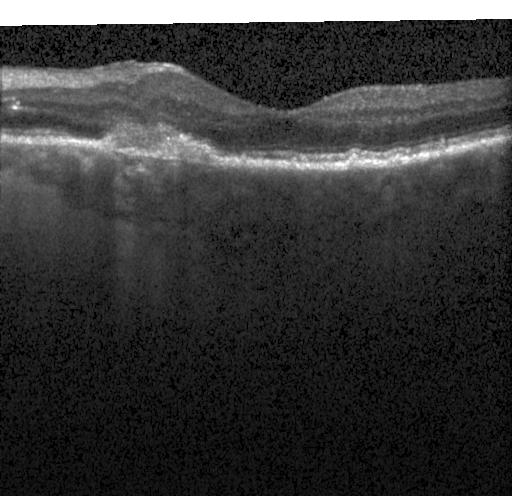 Horizontal scan through the fovea, spectral-domain OCT, OCT line scan, Heidelberg Spectralis — Diagnosis: CNV.